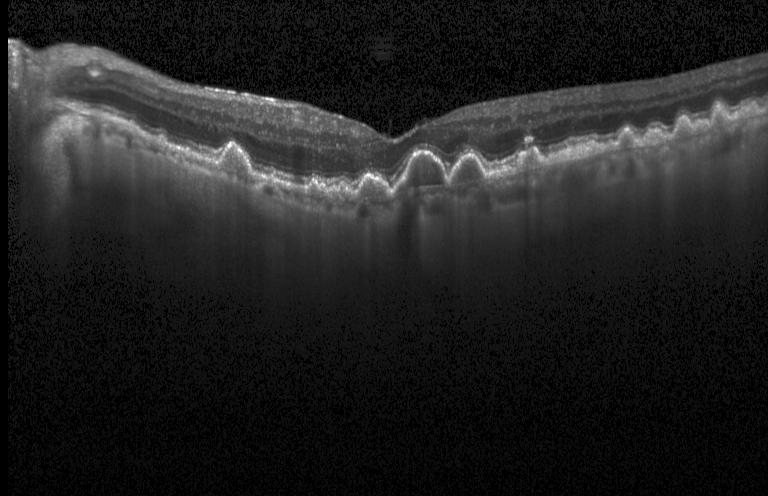

Spectral-domain OCT · OCT line scan.
Assessment: multiple drusen.